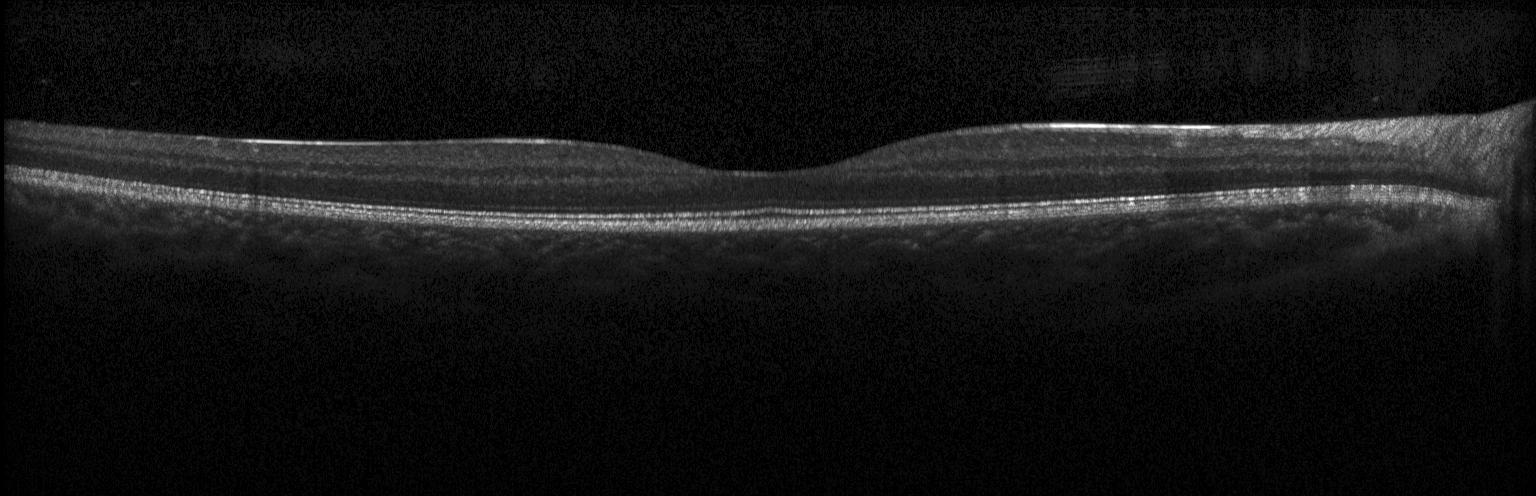

Retinal OCT B-scan · Heidelberg Spectralis · spectral-domain OCT. Impression: no choroidal neovascularization, diabetic macular edema, or drusen.